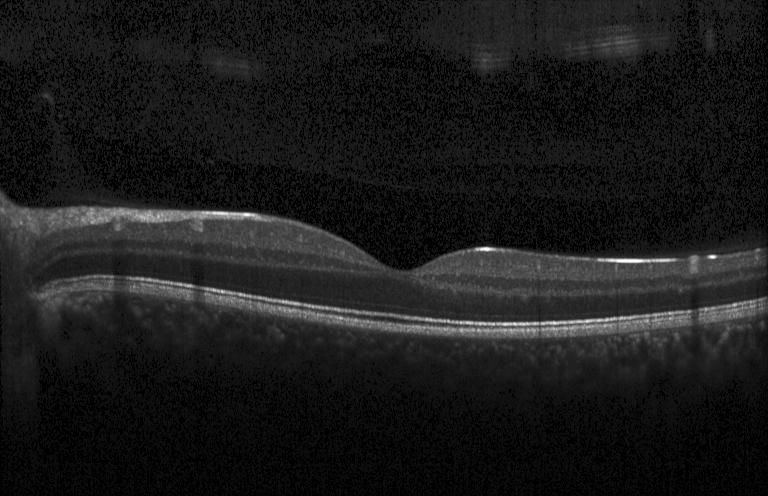
Impression: neither choroidal neovascularization, diabetic macular edema, nor drusen.